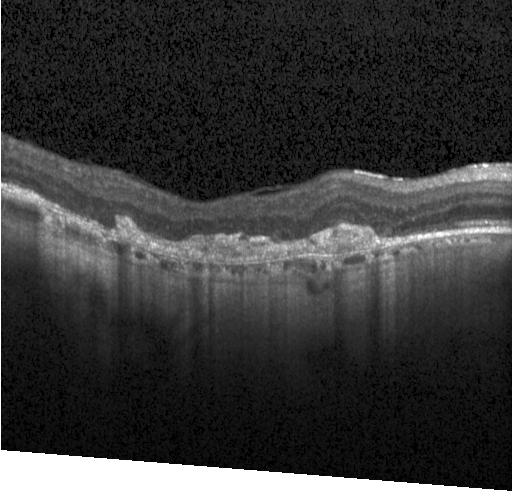 The scan shows a choroidal neovascular membrane.